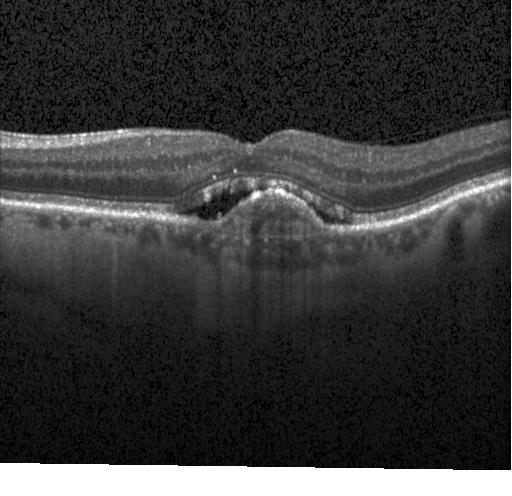

Spectral-domain OCT. Optical coherence tomography B-scan. A choroidal neovascular membrane.